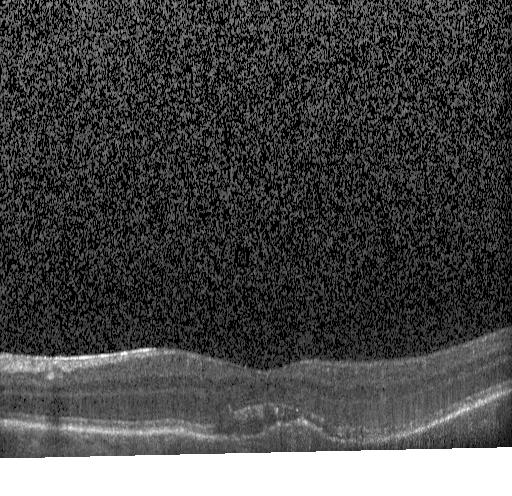
Impression: a choroidal neovascular membrane.